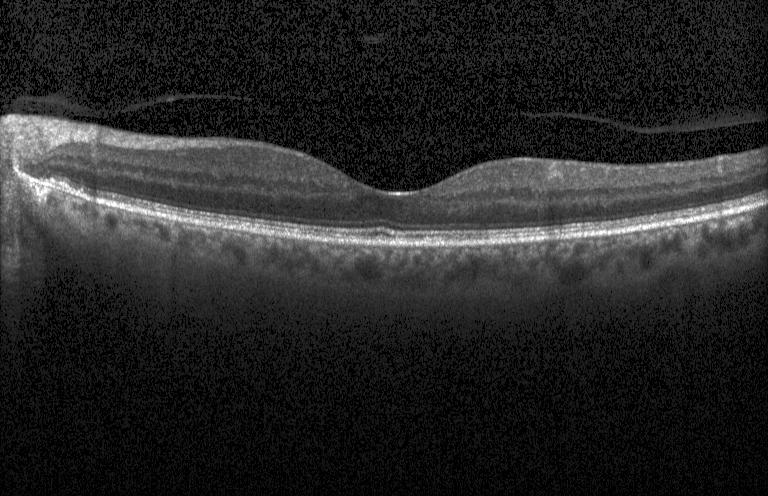
Macular scan · Heidelberg Spectralis OCT system · SD-OCT · OCT B-scan. Diagnosis: no evidence of CNV, DME, or drusen.